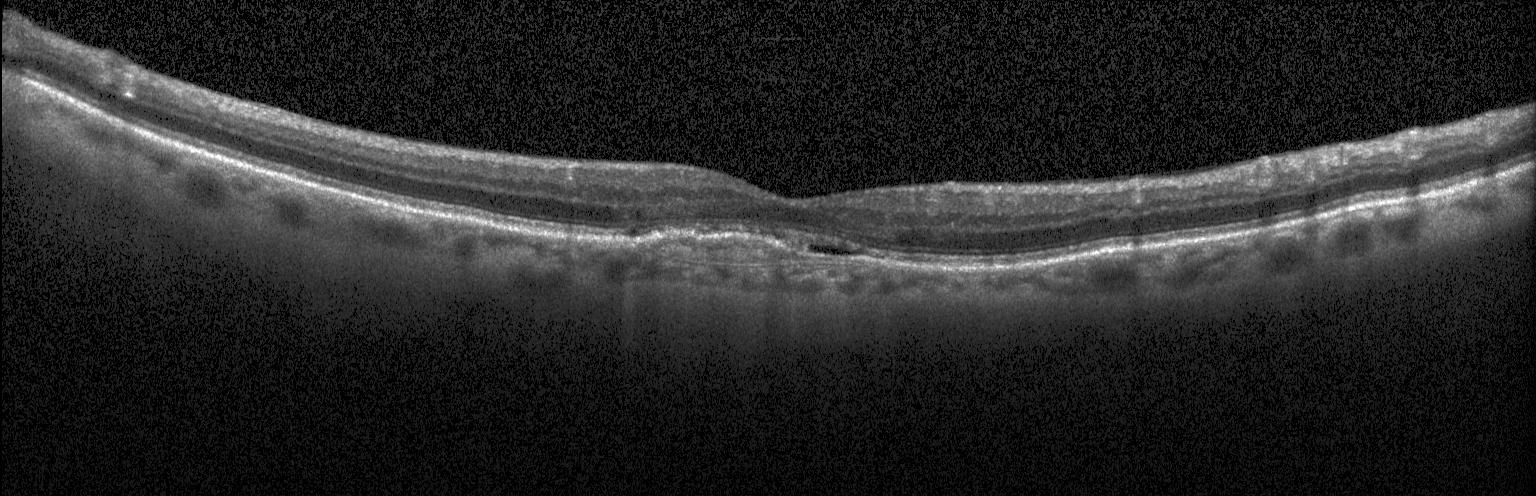

Spectral-domain optical coherence tomography. Heidelberg Spectralis OCT system. Retinal OCT cross-section. Through the macula.
Impression: a choroidal neovascular membrane.